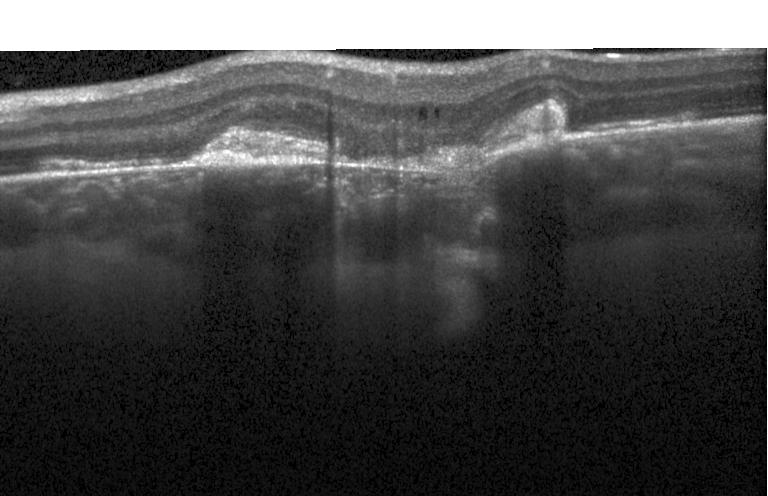 Instrument: Heidelberg Spectralis · optical coherence tomography scan · SD-OCT · horizontal scan through the fovea.
Diagnosis: a choroidal neovascular membrane.